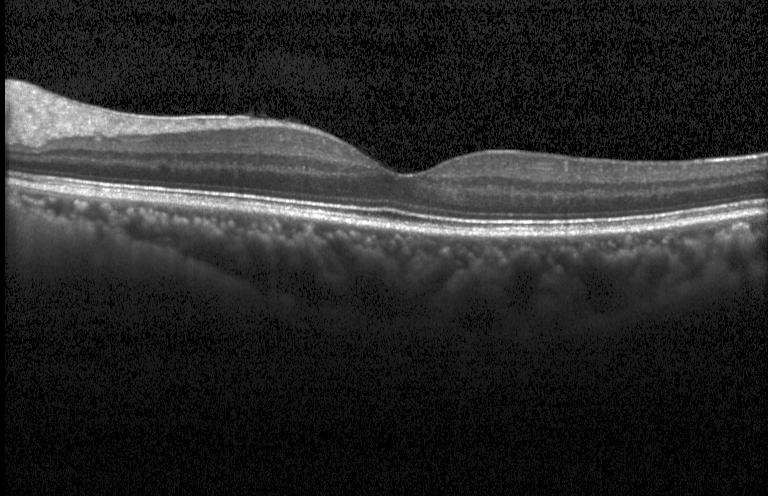 Horizontal scan through the fovea; optical coherence tomography scan.
Impression: no choroidal neovascularization, no diabetic macular edema, and no drusen.